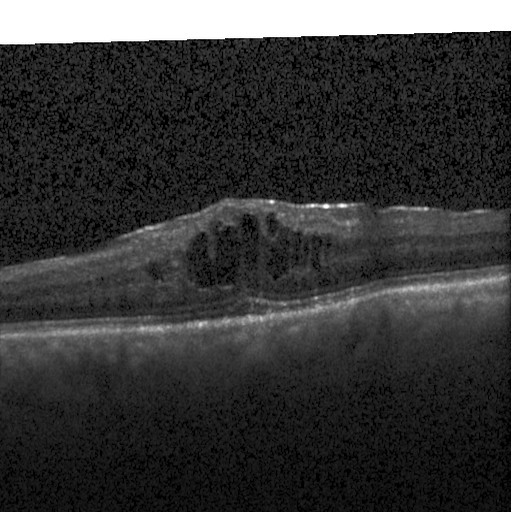 Fovea-centered · OCT B-scan.
Finding: DME.